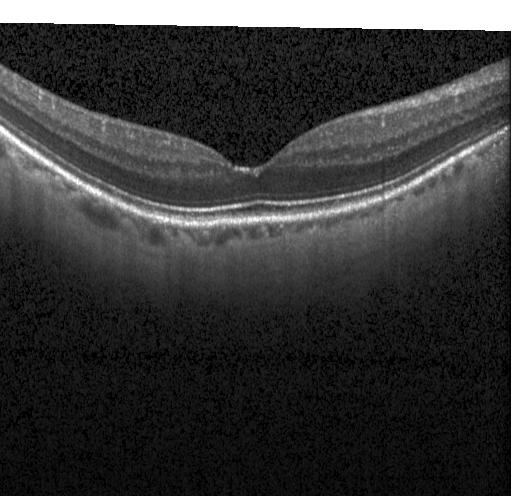

Optical coherence tomography scan · fovea-centered. The scan shows no choroidal neovascularization, diabetic macular edema, or drusen.